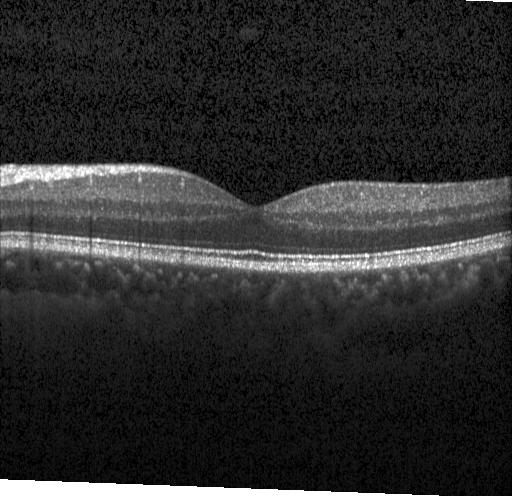 Macular OCT demonstrating no evidence of CNV, DME, or drusen.